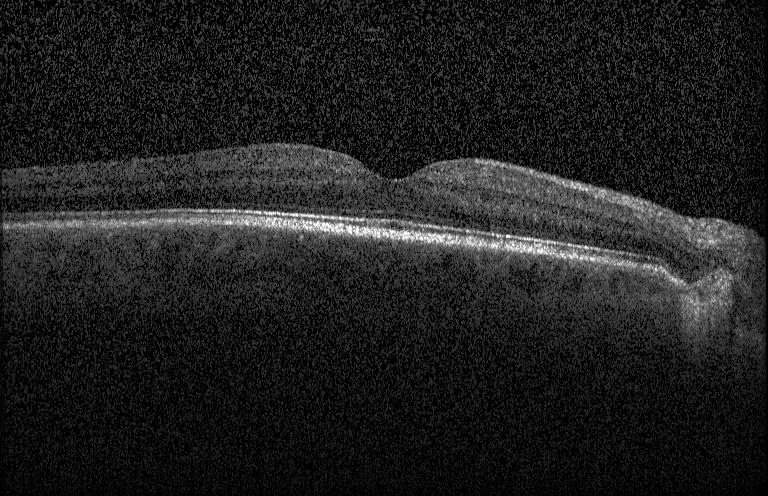 Retinal OCT cross-section showing no CNV, no DME, and no drusen.